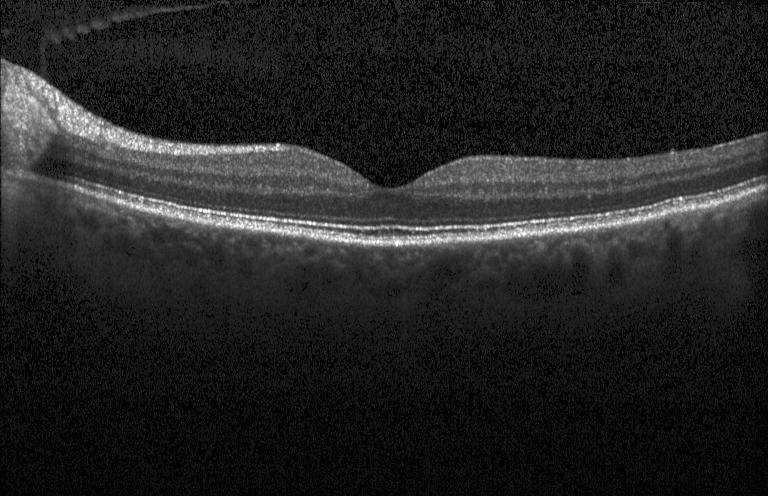
Through the macula. Spectral-domain optical coherence tomography. Acquired on a Heidelberg Spectralis. Optical coherence tomography scan — OCT finding: no choroidal neovascularization, diabetic macular edema, or drusen.